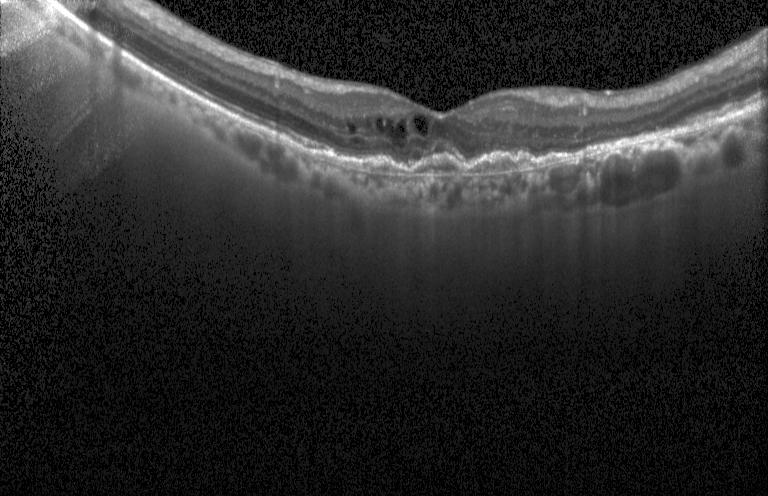

Retinal OCT cross-section; Heidelberg Spectralis OCT system; horizontal scan through the fovea; spectral-domain optical coherence tomography. Diagnosis: a choroidal neovascular membrane.